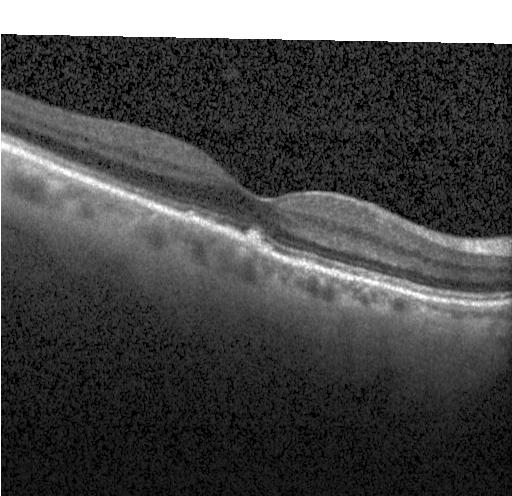

OCT finding: drusen.